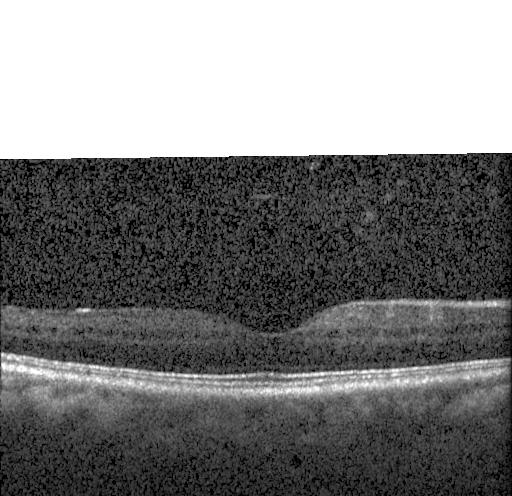

Macular OCT demonstrating no CNV, no DME, and no drusen.